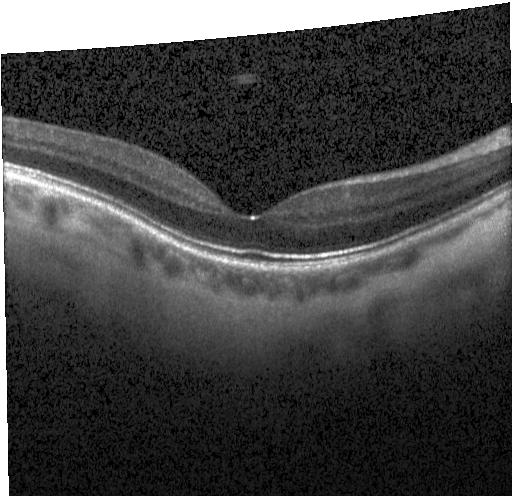 Heidelberg Spectralis. Spectral-domain optical coherence tomography. Optical coherence tomography B-scan. Fovea-centered. Impression: no choroidal neovascularization, no diabetic macular edema, and no drusen.